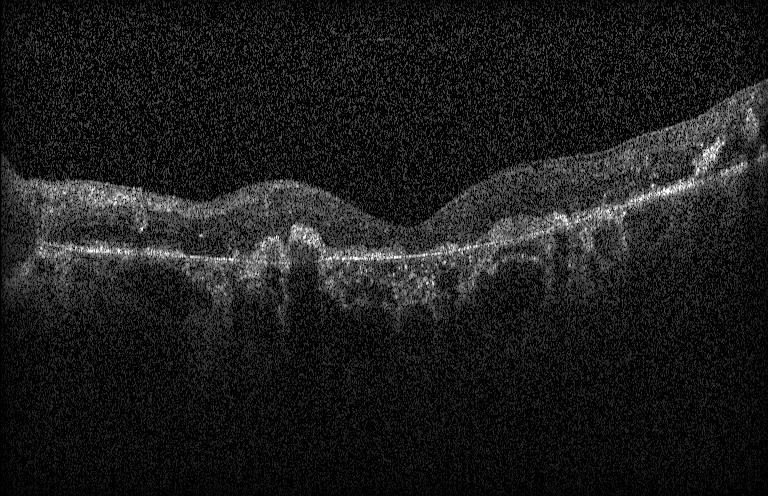
Impression: a choroidal neovascular membrane.